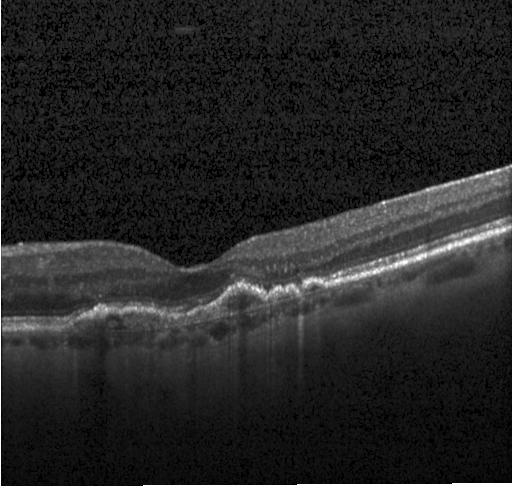 Diagnosis: choroidal neovascularization.